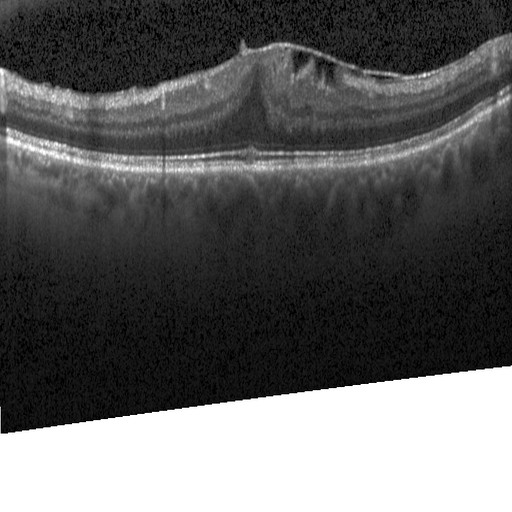

Retinal OCT B-scan · spectral-domain optical coherence tomography — Assessment: DME.